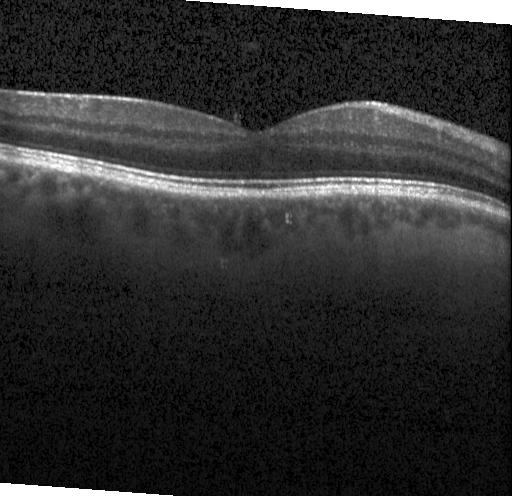 OCT finding: no CNV, no DME, and no drusen.